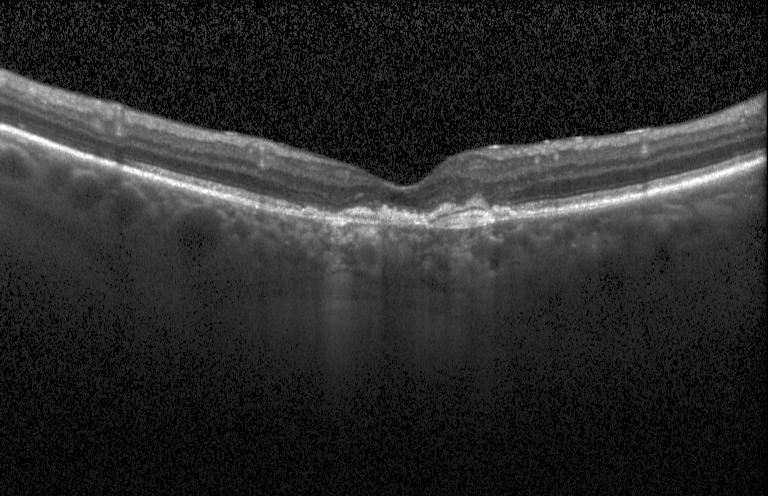

OCT B-scan. A choroidal neovascular membrane.